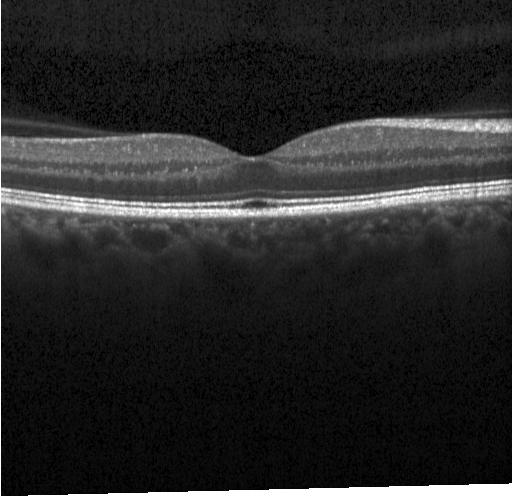 Macular scan; SD-OCT; retinal OCT cross-section.
Impression: no CNV, DME, or drusen.